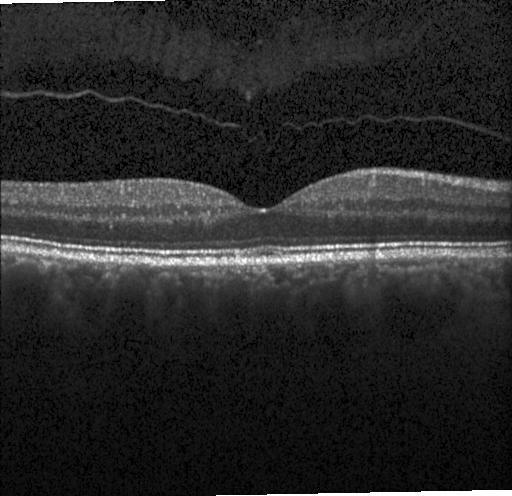
Heidelberg Spectralis OCT system; spectral-domain OCT; retinal OCT B-scan.
No choroidal neovascularization, diabetic macular edema, or drusen.